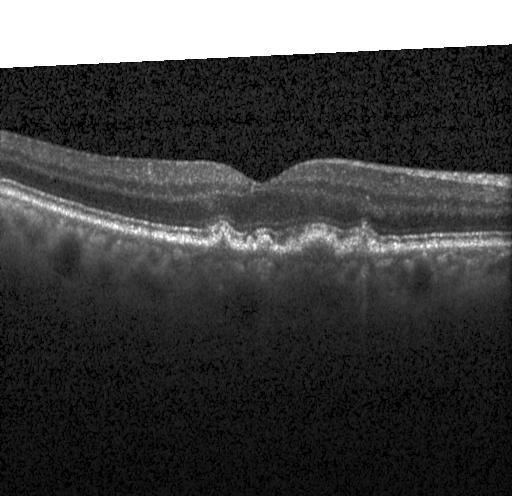
Acquired on a Heidelberg Spectralis, centered on the fovea, optical coherence tomography B-scan
Impression: sub-RPE drusenoid deposits.